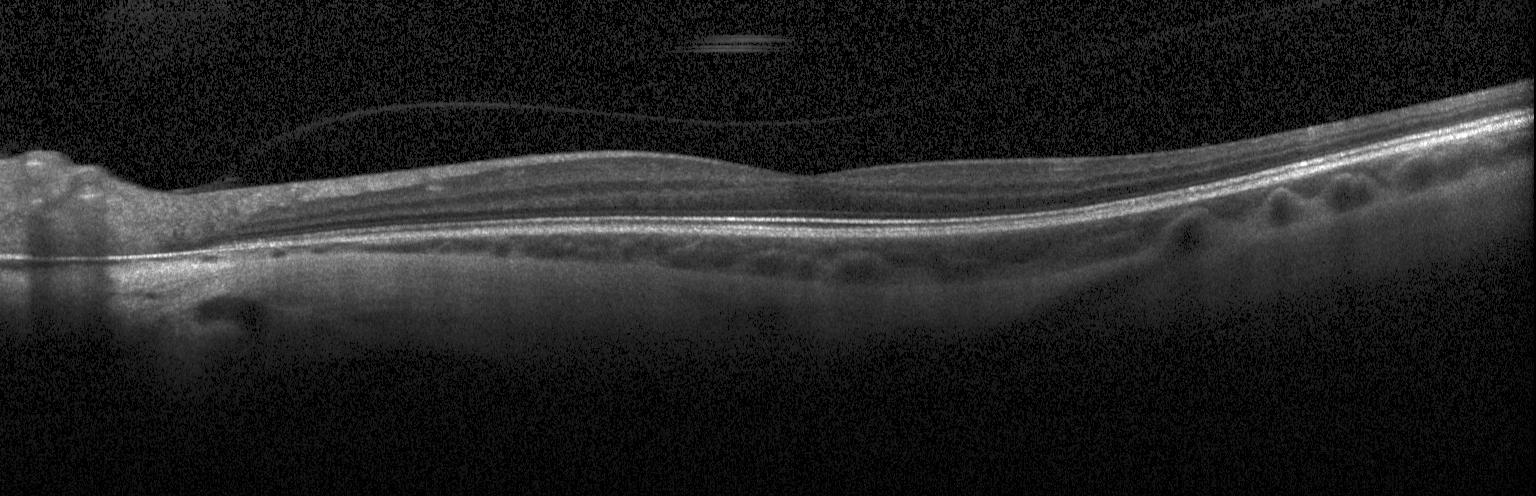 Optical coherence tomography scan.
This B-scan demonstrates no evidence of CNV, DME, or drusen.